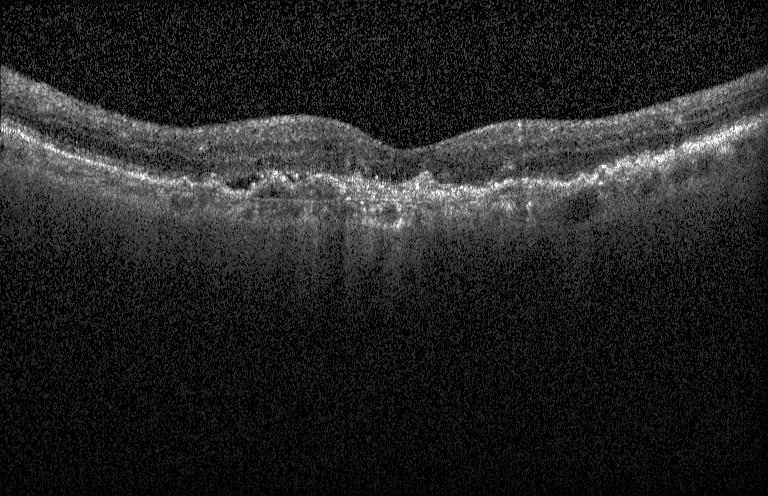 OCT line scan. Through the macula.
Diagnosis: a choroidal neovascular membrane.